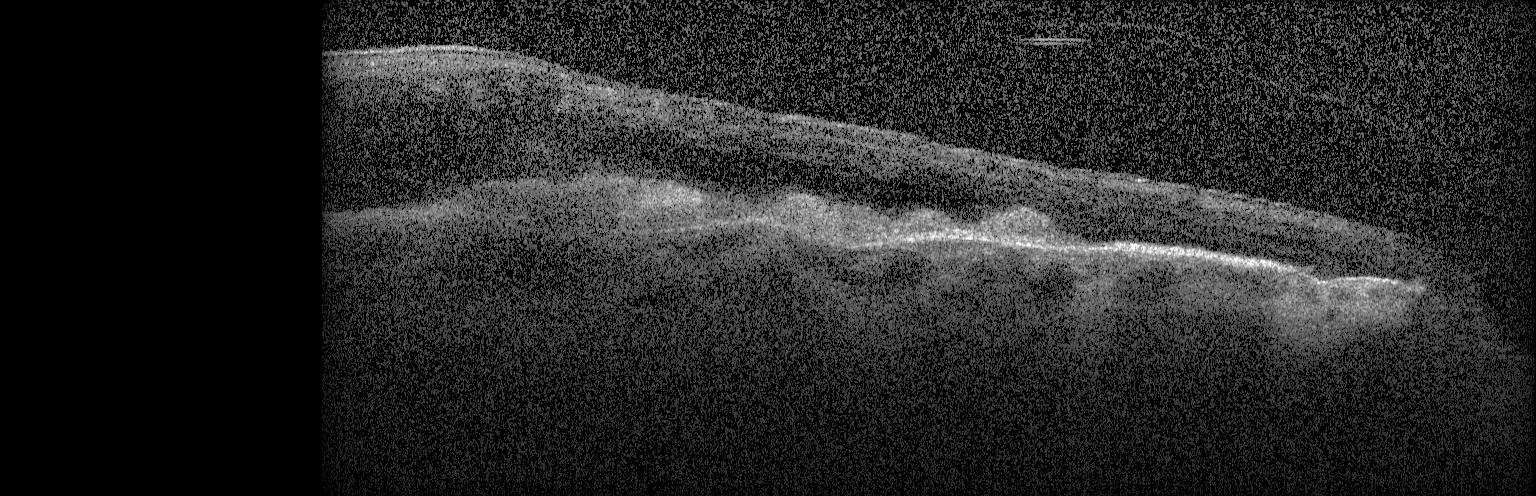
The scan shows a choroidal neovascular membrane.